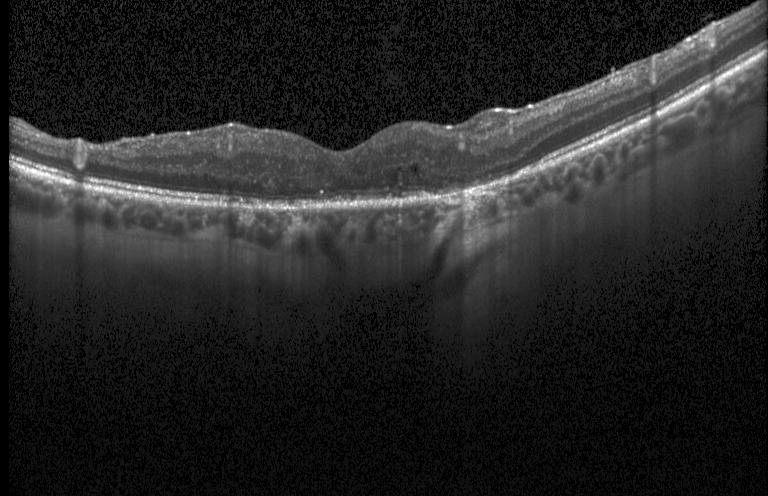

Finding: diabetic macular edema (DME).